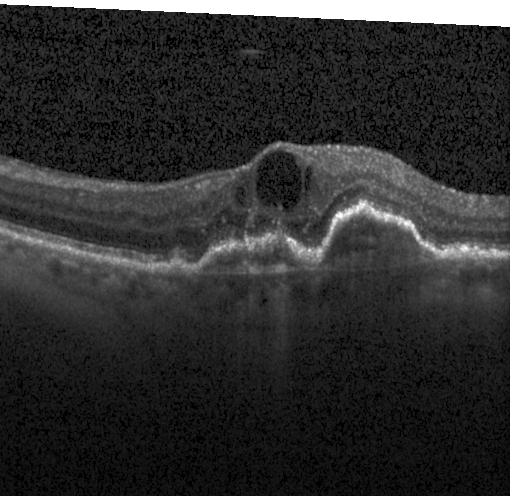

SD-OCT; instrument: Heidelberg Spectralis; through the macula; optical coherence tomography B-scan.
Assessment: choroidal neovascularization (CNV).